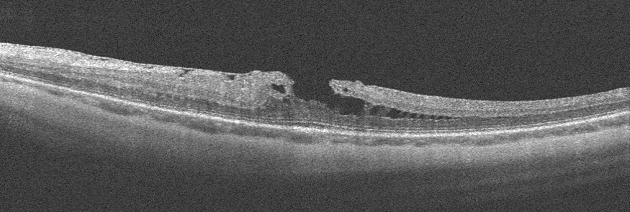
OCT B-scan · left eye. This B-scan demonstrates vitreomacular interface disease.